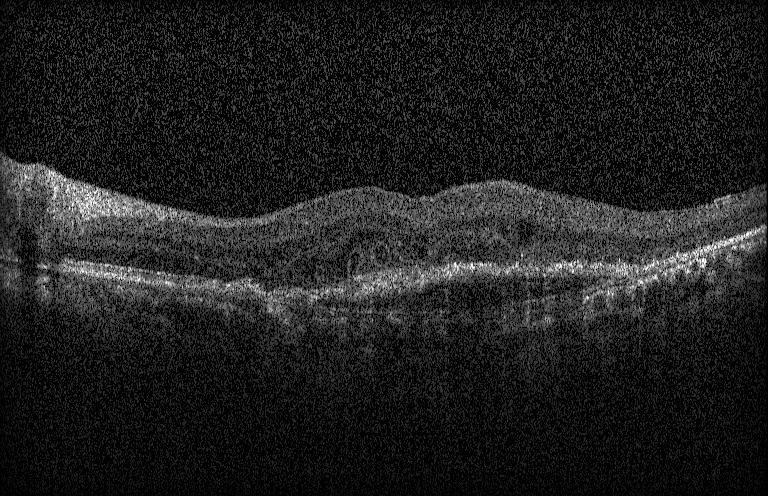
SD-OCT · retinal OCT cross-section
Assessment: a choroidal neovascular membrane.